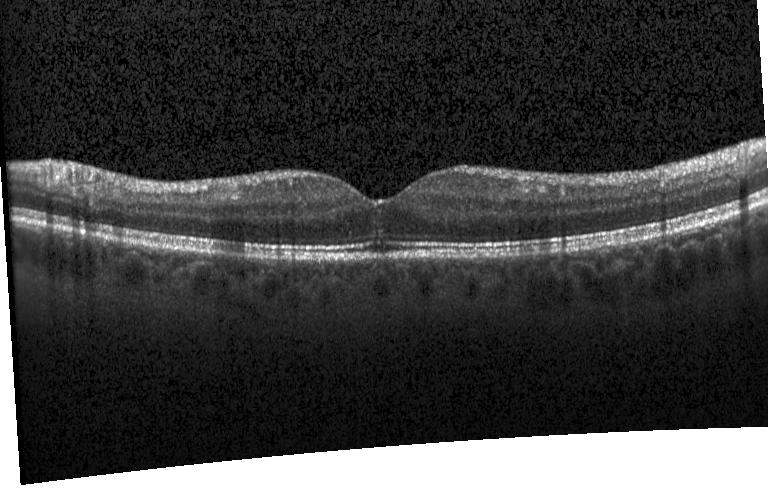
The scan shows no choroidal neovascularization, diabetic macular edema, or drusen.